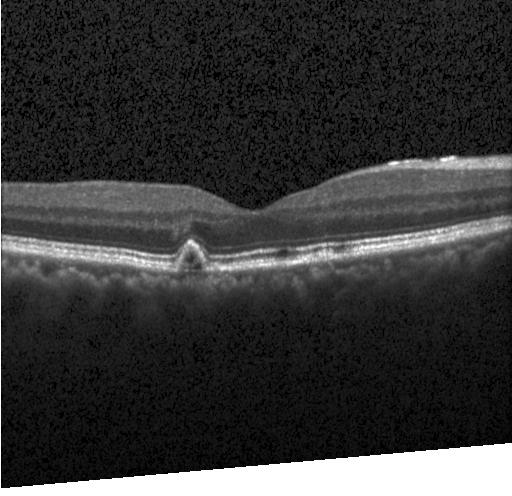
The scan shows multiple drusen.